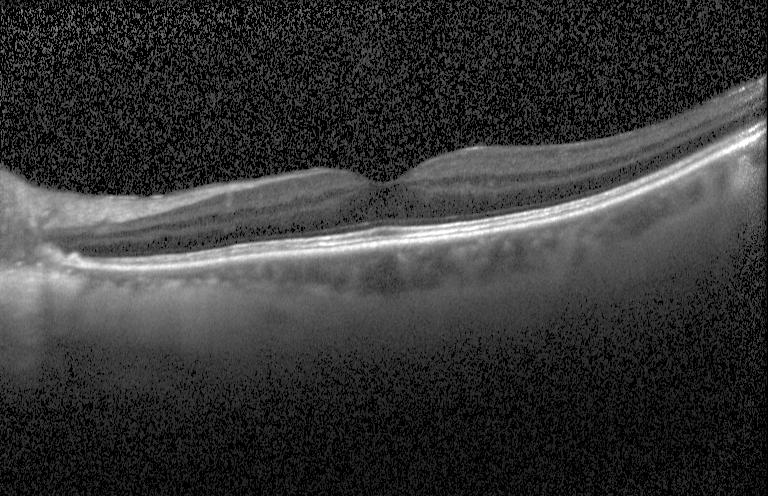 No CNV, DME, or drusen.